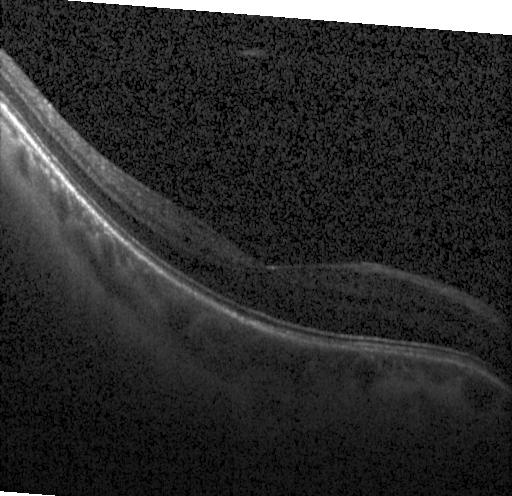
Spectral-domain OCT. Instrument: Heidelberg Spectralis. Optical coherence tomography B-scan. Macular scan.
Finding: no choroidal neovascularization, diabetic macular edema, or drusen.